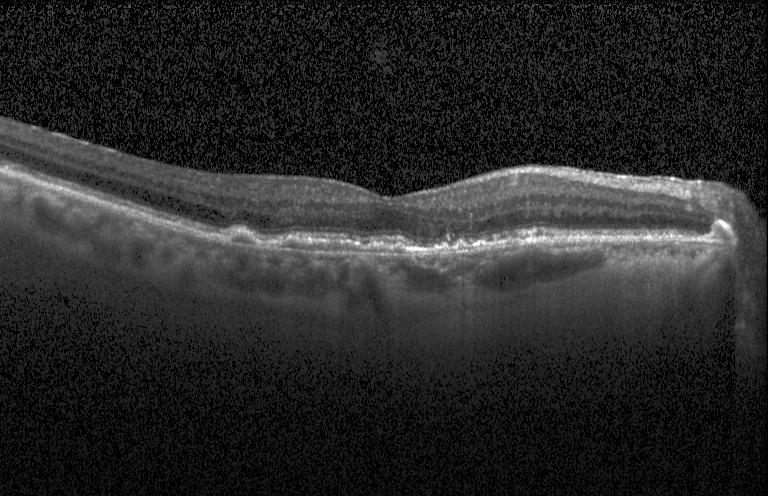 Centered on the fovea. SD-OCT. Acquired on a Heidelberg Spectralis. OCT B-scan
This B-scan demonstrates a choroidal neovascular membrane.